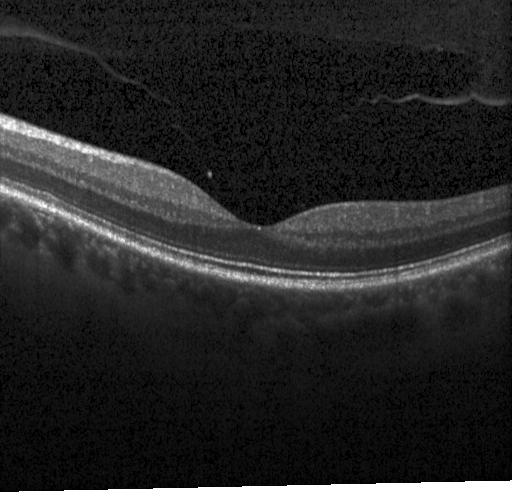
Centered on the fovea · OCT B-scan · instrument: Heidelberg Spectralis — Finding: no choroidal neovascularization, no diabetic macular edema, and no drusen.